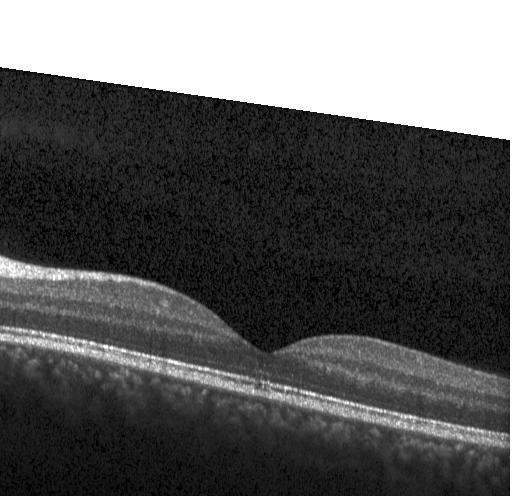

Through the macula, Heidelberg Spectralis OCT system, spectral-domain OCT, retinal OCT cross-section.
Macular OCT: neither choroidal neovascularization, diabetic macular edema, nor drusen.